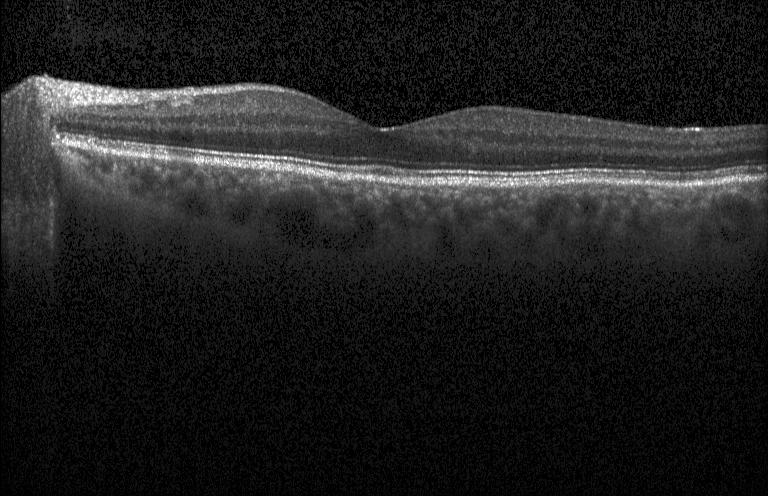 The scan shows no choroidal neovascularization, diabetic macular edema, or drusen.